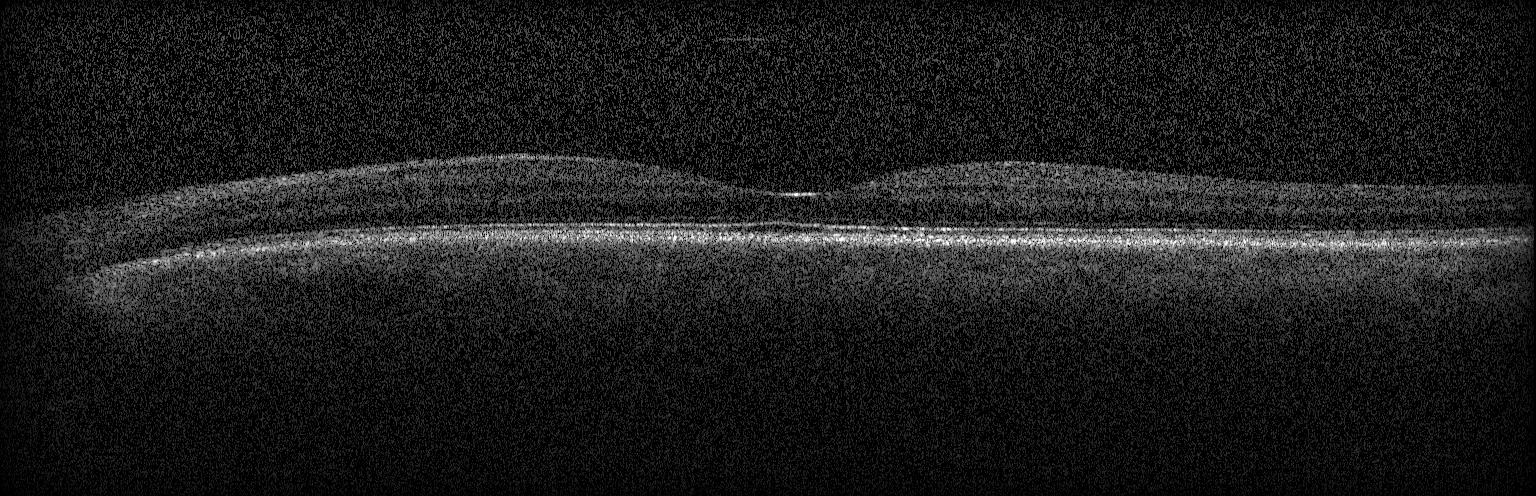
Retinal OCT B-scan · macular scan
This B-scan demonstrates neither choroidal neovascularization, diabetic macular edema, nor drusen.